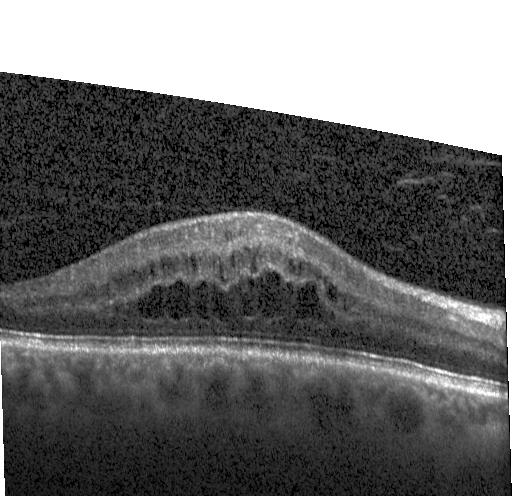 Finding: diabetic macular edema.